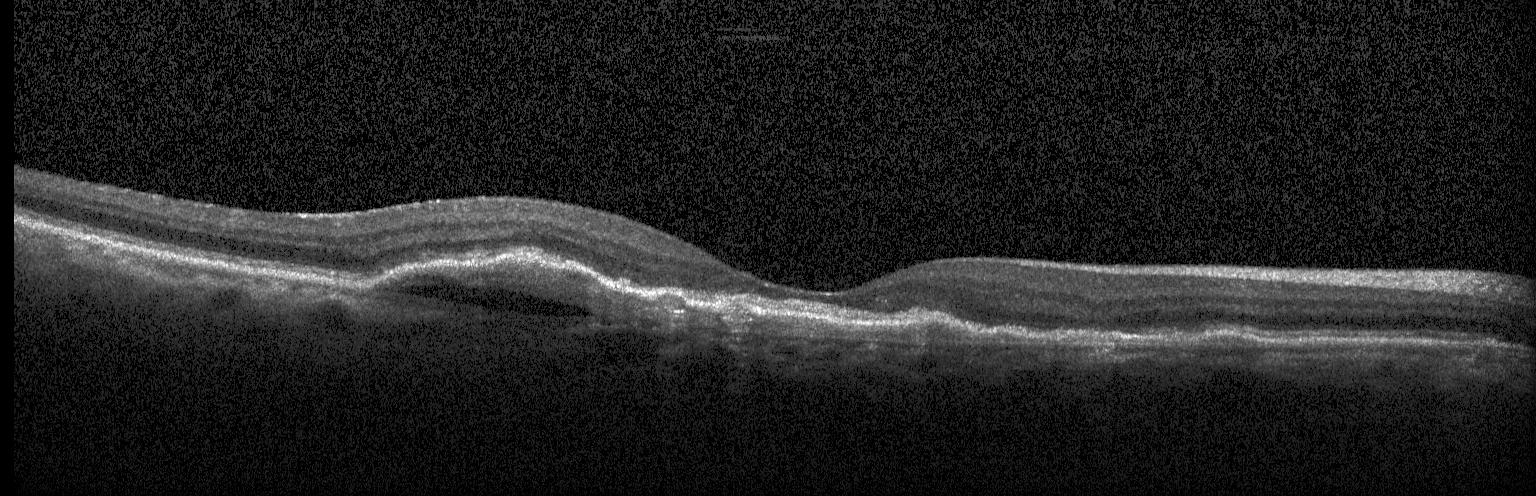 Acquired on a Heidelberg Spectralis · SD-OCT · fovea-centered · optical coherence tomography B-scan. Diagnosis: CNV.